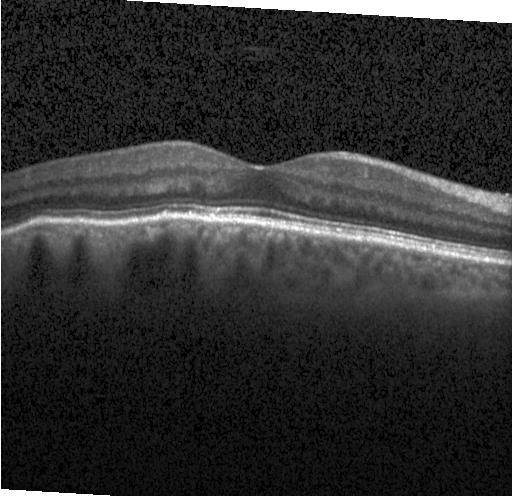 OCT line scan.
Impression: no evidence of CNV, DME, or drusen.